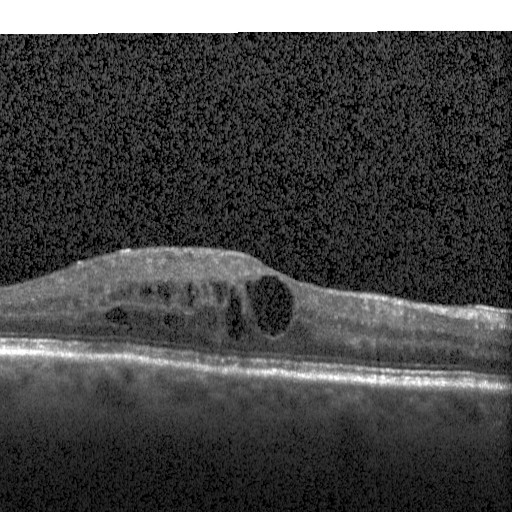

Heidelberg Spectralis OCT system · spectral-domain optical coherence tomography · optical coherence tomography B-scan · through the macula — Diabetic macular edema (DME).